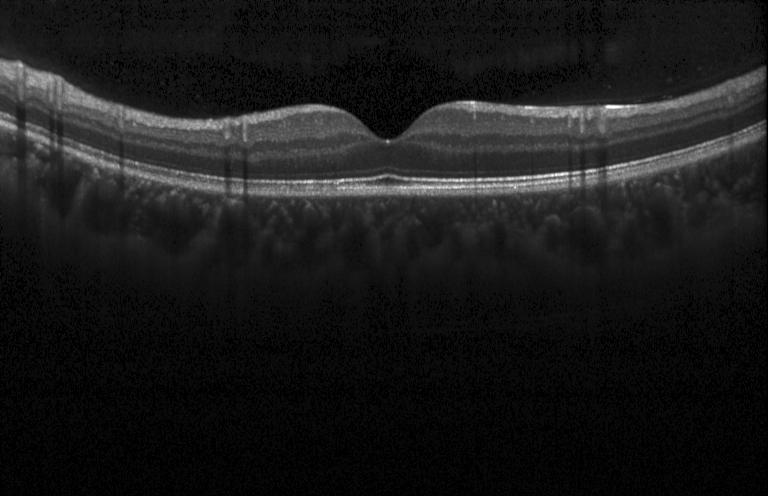
Dx: neither CNV, DME, nor drusen.